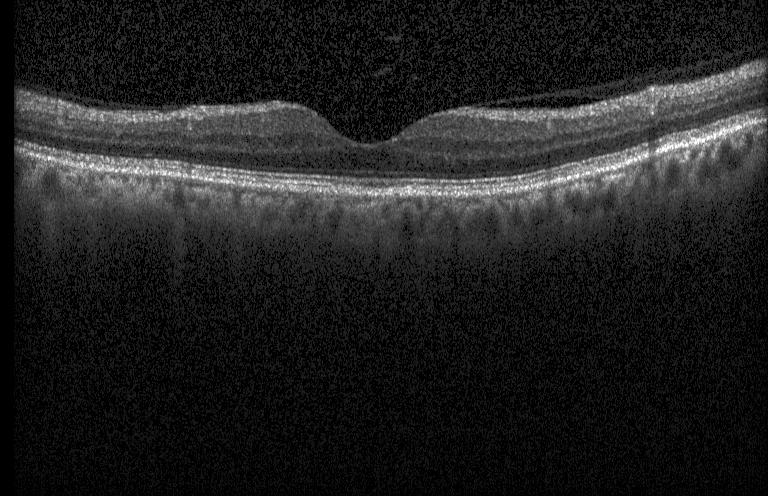

Through the macula. Retinal OCT cross-section. Instrument: Heidelberg Spectralis. Dx: neither choroidal neovascularization, diabetic macular edema, nor drusen.